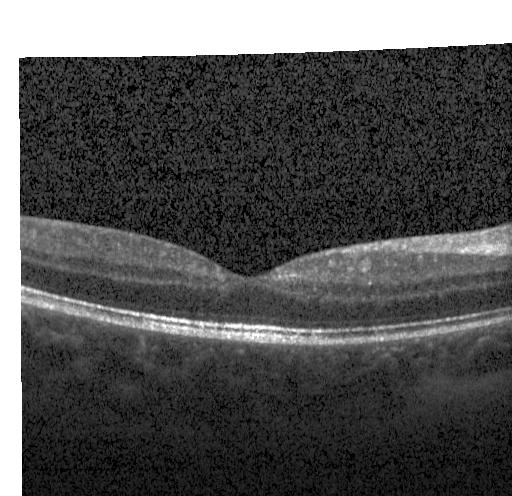

OCT B-scan.
The scan shows no evidence of CNV, DME, or drusen.